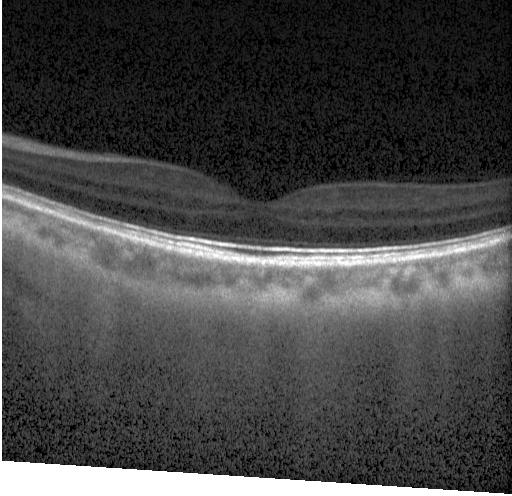
Acquired on a Heidelberg Spectralis; centered on the fovea; SD-OCT; retinal OCT cross-section
Finding: neither CNV, DME, nor drusen.